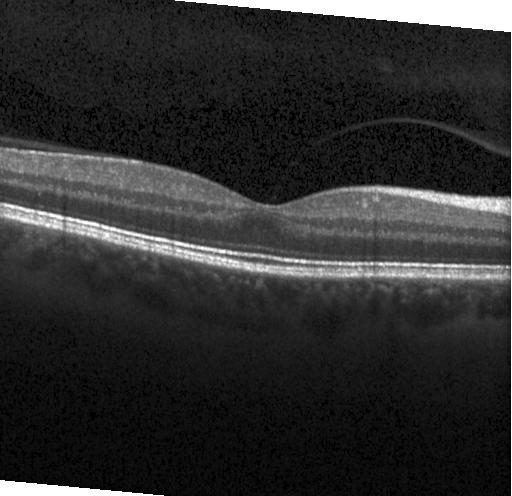 The scan shows no evidence of CNV, DME, or drusen.